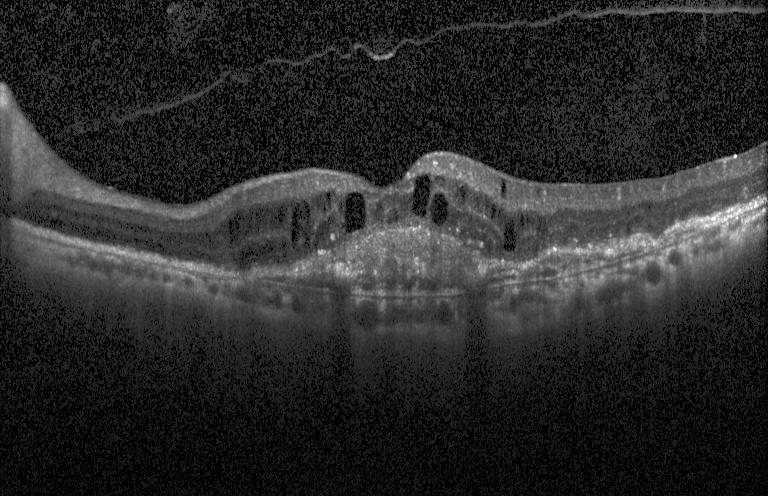 Finding: a choroidal neovascular membrane.